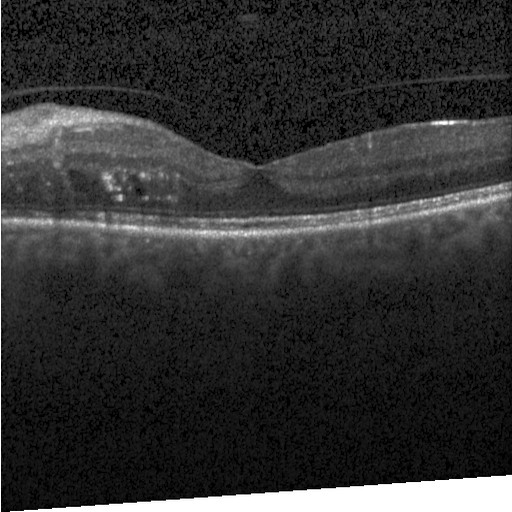

Spectral-domain optical coherence tomography · acquired on a Heidelberg Spectralis · centered on the fovea · optical coherence tomography B-scan.
Diagnosis: DME.